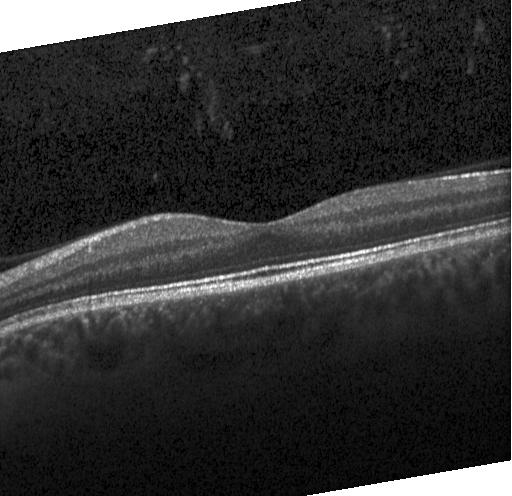

Retinal OCT B-scan
Dx: no choroidal neovascularization, no diabetic macular edema, and no drusen.